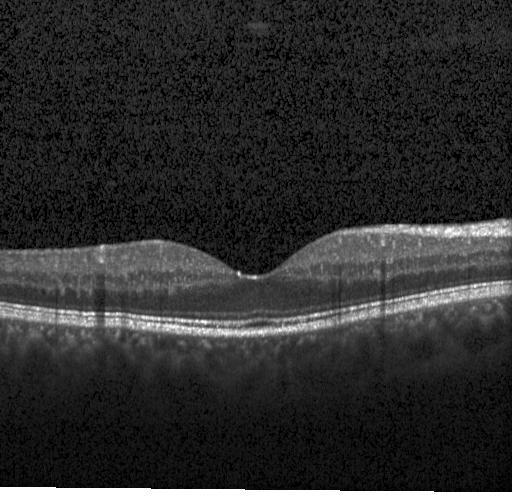
Retinal OCT B-scan. Spectral-domain optical coherence tomography. Centered on the fovea. Heidelberg Spectralis
Diagnosis: no choroidal neovascularization, diabetic macular edema, or drusen.